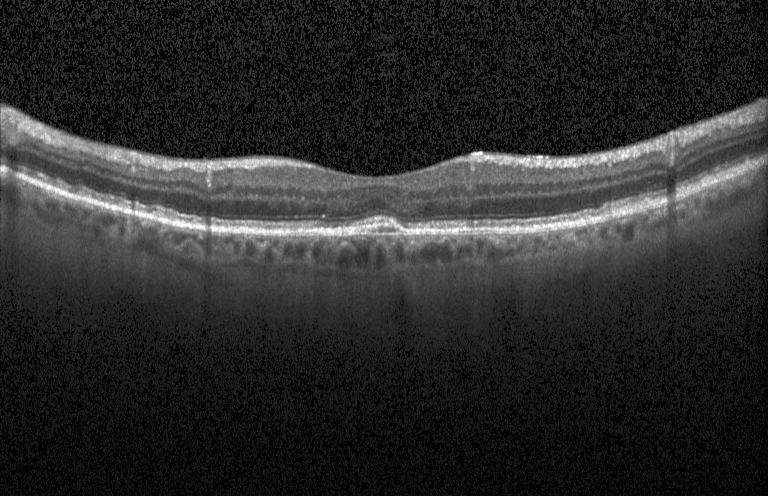
OCT line scan, instrument: Heidelberg Spectralis — Finding: drusen.